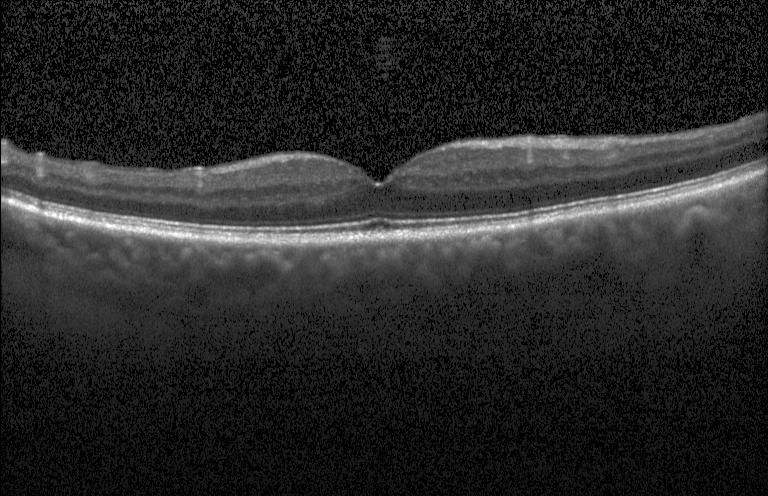

Horizontal scan through the fovea, optical coherence tomography B-scan, spectral-domain optical coherence tomography.
Dx: neither CNV, DME, nor drusen.